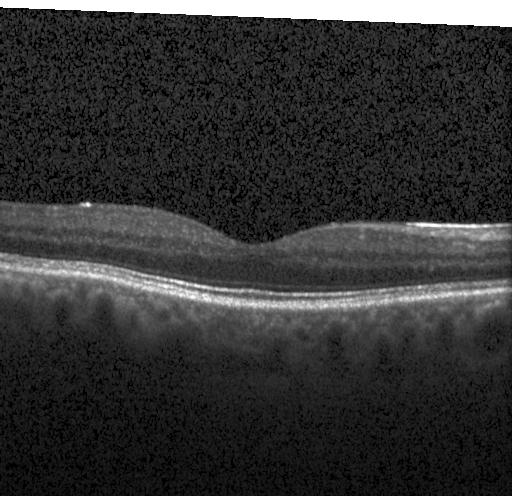
Optical coherence tomography scan
Assessment: no evidence of CNV, DME, or drusen.